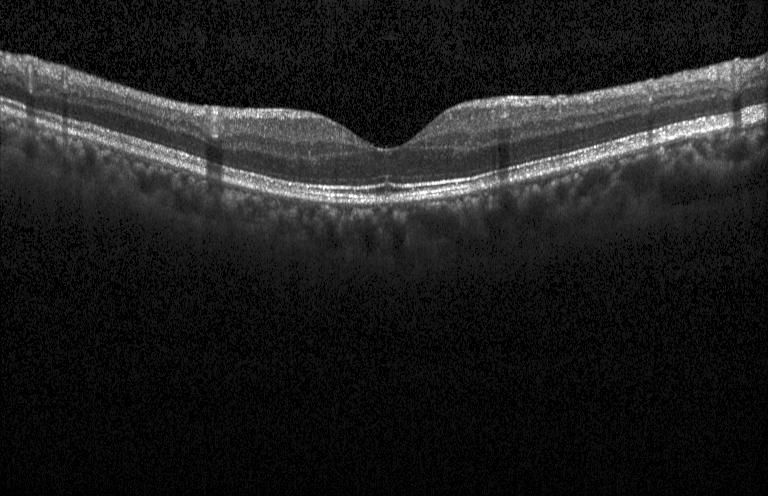
Optical coherence tomography scan. Spectral-domain OCT
Diagnosis: neither choroidal neovascularization, diabetic macular edema, nor drusen.